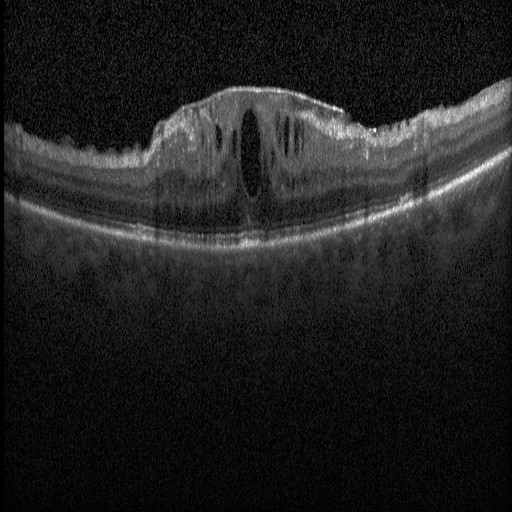 Optical coherence tomography B-scan, horizontal scan through the fovea, Heidelberg Spectralis OCT system
Macular OCT: diabetic macular edema.